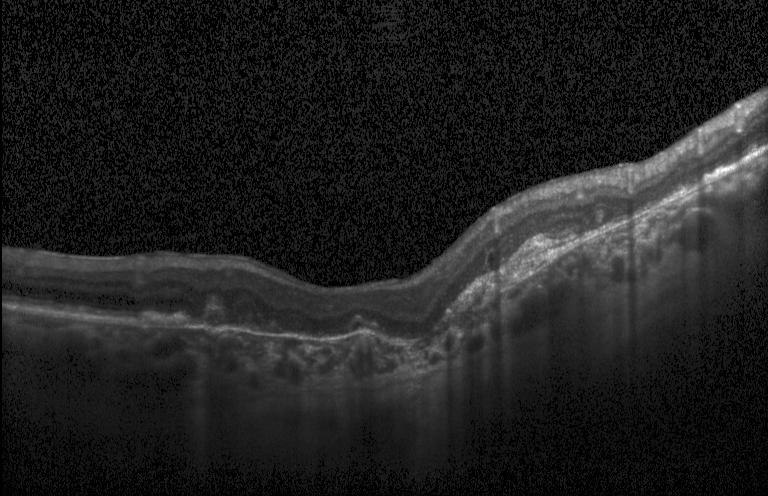 Optical coherence tomography scan
Diagnosis: a choroidal neovascular membrane.